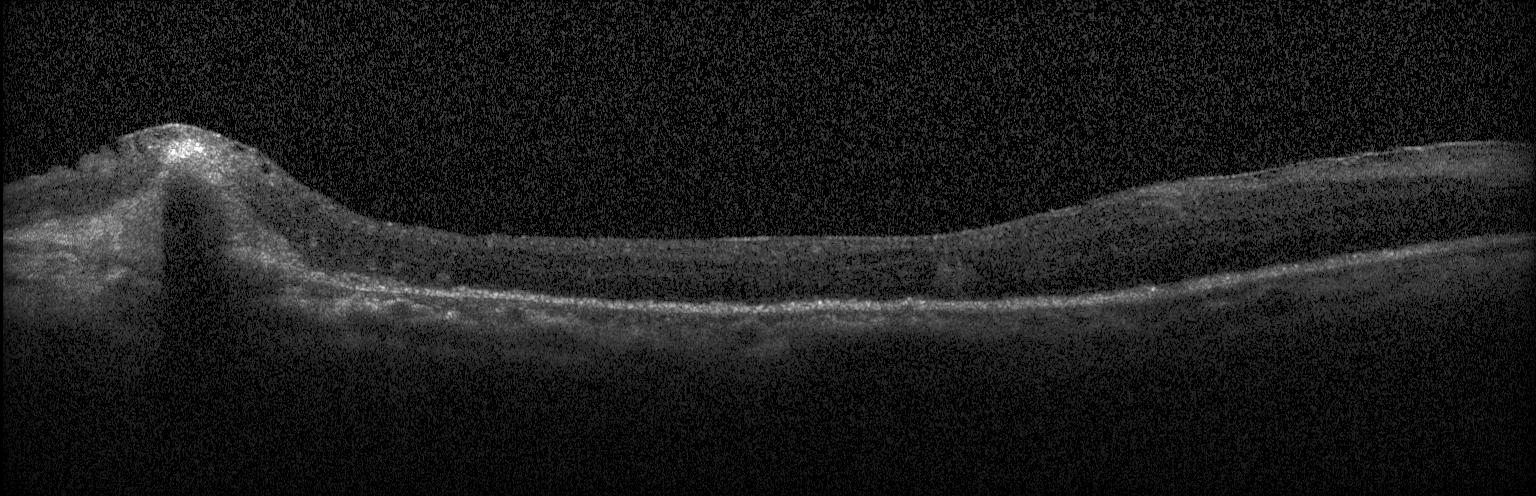 Acquired on a Heidelberg Spectralis · optical coherence tomography B-scan.
This B-scan demonstrates a choroidal neovascular membrane.